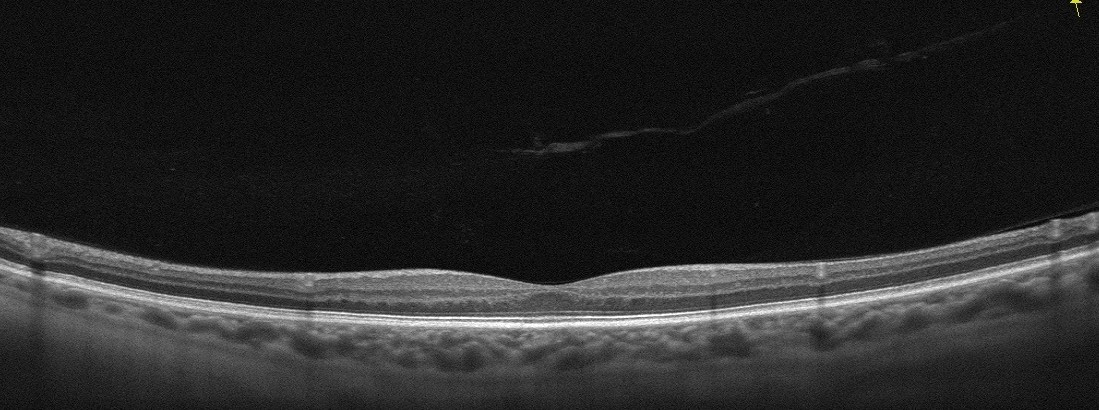
Finding: no AMD, DME, ERM, RAO, RVO, or VID.